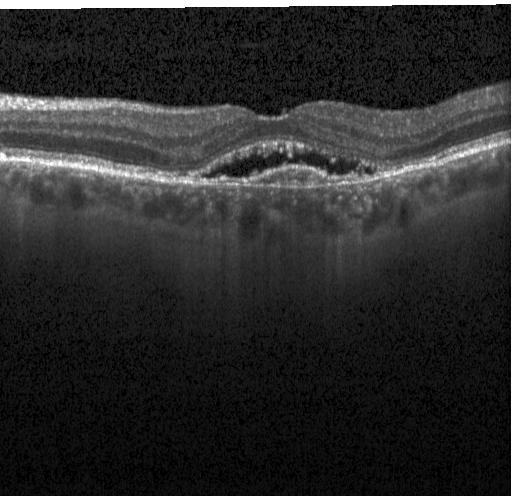 OCT B-scan
Assessment: a choroidal neovascular membrane.